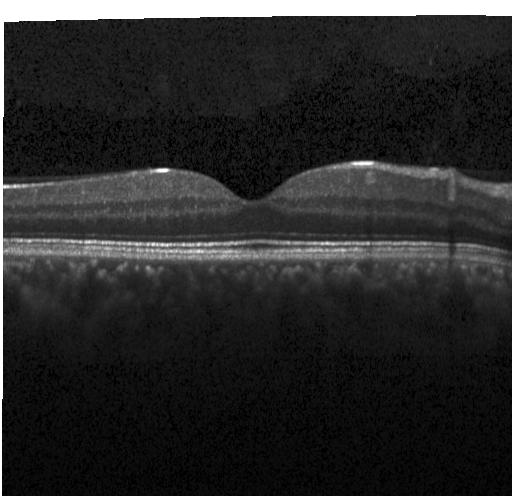
Diagnosis: no evidence of choroidal neovascularization, diabetic macular edema, or drusen.